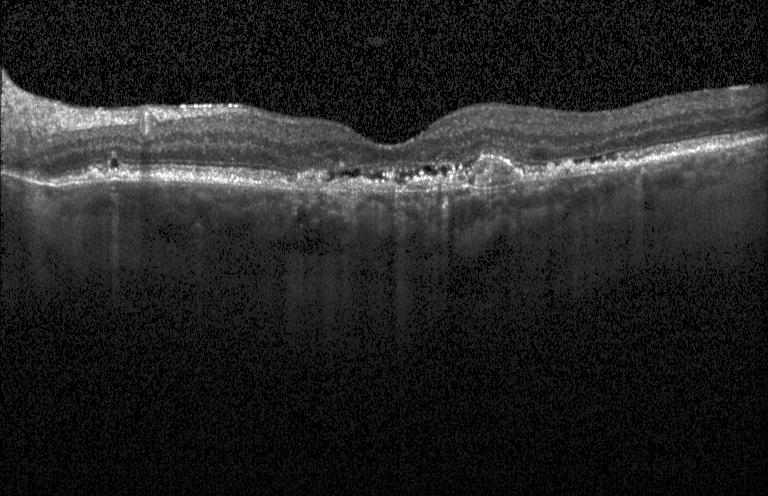
Heidelberg Spectralis OCT system. OCT line scan. Fovea-centered. SD-OCT.
A choroidal neovascular membrane.